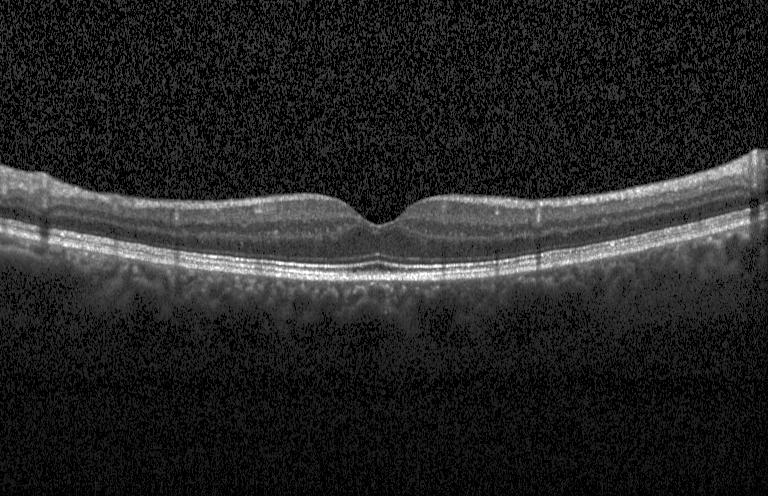
Optical coherence tomography scan. Instrument: Heidelberg Spectralis. Impression: no choroidal neovascularization, diabetic macular edema, or drusen.